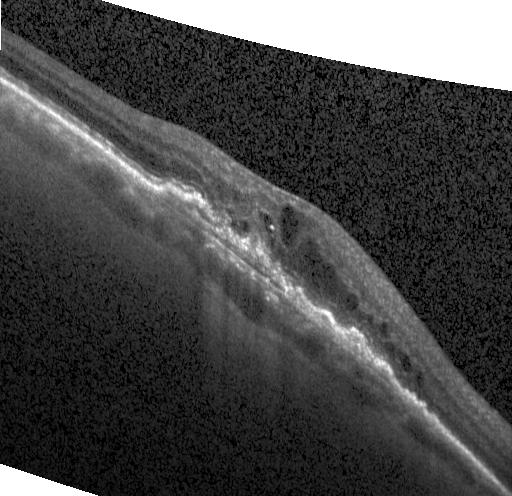
Horizontal scan through the fovea; spectral-domain OCT; OCT B-scan; acquired on a Heidelberg Spectralis — Dx: CNV.